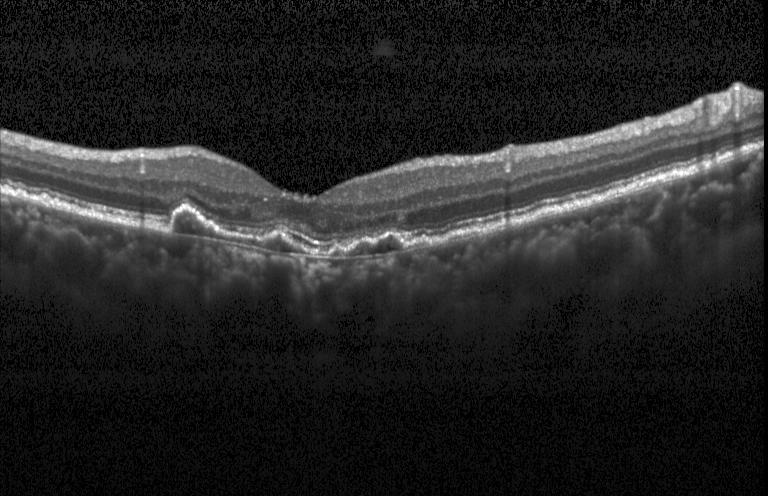 Fovea-centered; Heidelberg Spectralis; spectral-domain OCT; optical coherence tomography B-scan.
Finding: choroidal neovascularization (CNV).